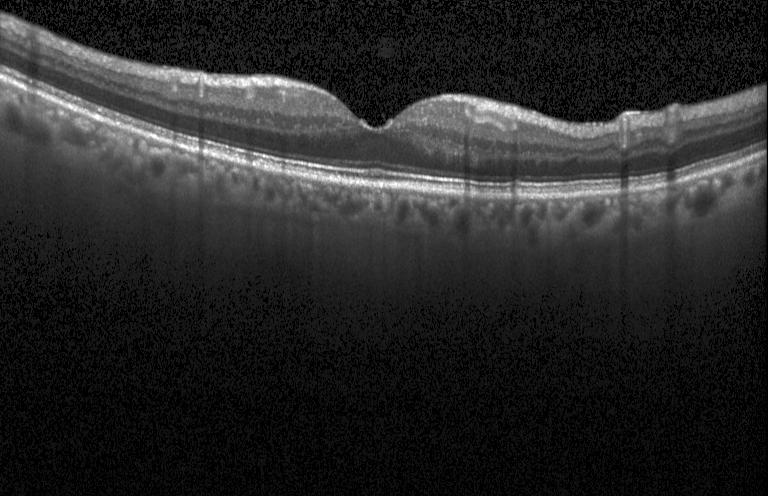 Optical coherence tomography B-scan; centered on the fovea; acquired on a Heidelberg Spectralis. The scan shows no evidence of choroidal neovascularization, diabetic macular edema, or drusen.